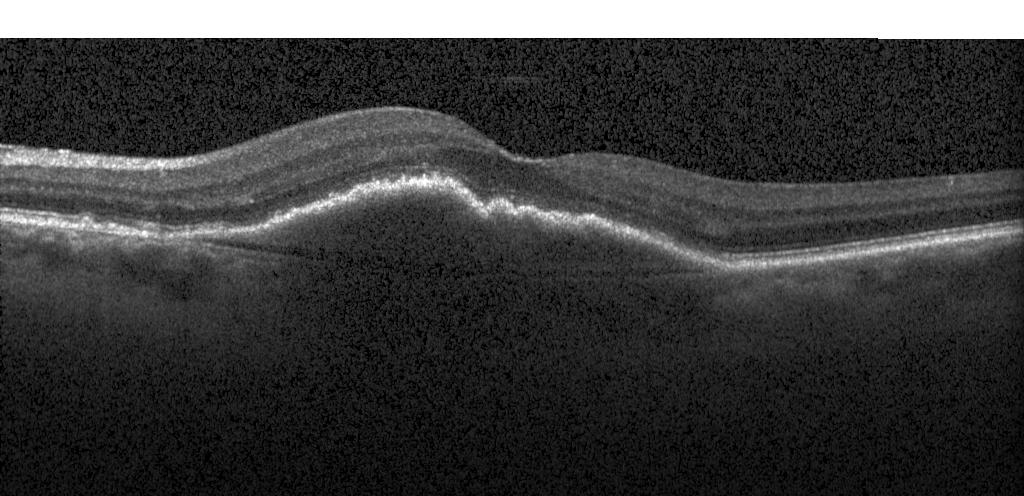 Retinal OCT B-scan — Impression: CNV.